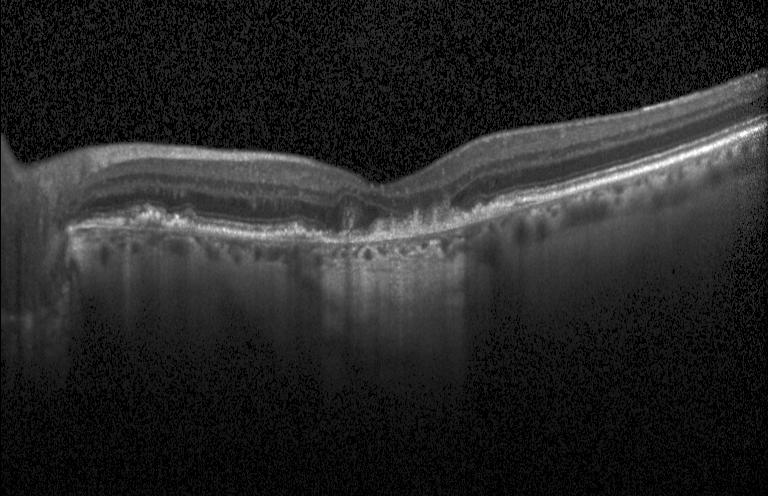 OCT line scan. Finding: CNV.